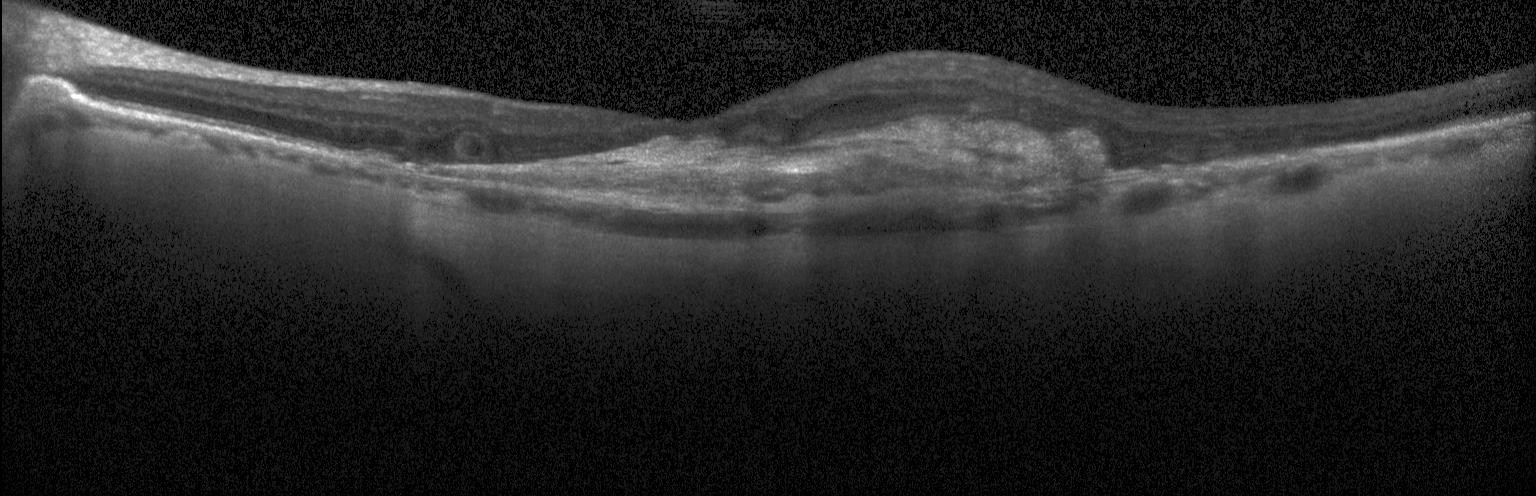

Heidelberg Spectralis, SD-OCT, macular scan, retinal OCT cross-section.
Finding: a choroidal neovascular membrane.